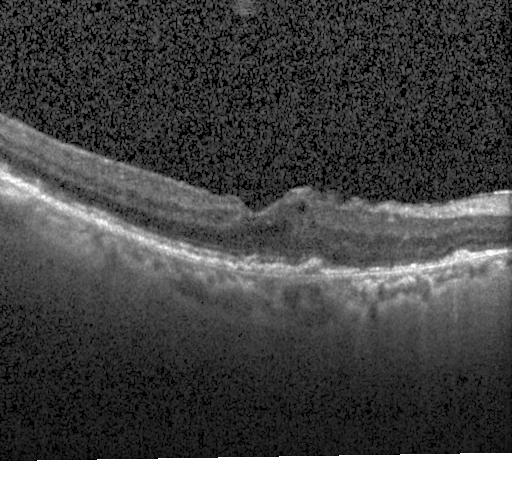 Diagnosis: choroidal neovascularization (CNV).